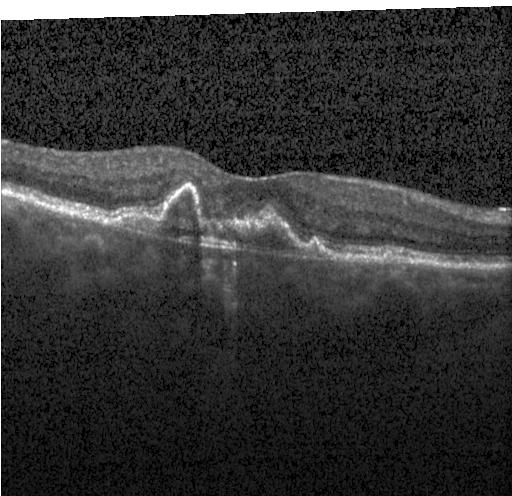

Diagnosis: choroidal neovascularization (CNV).